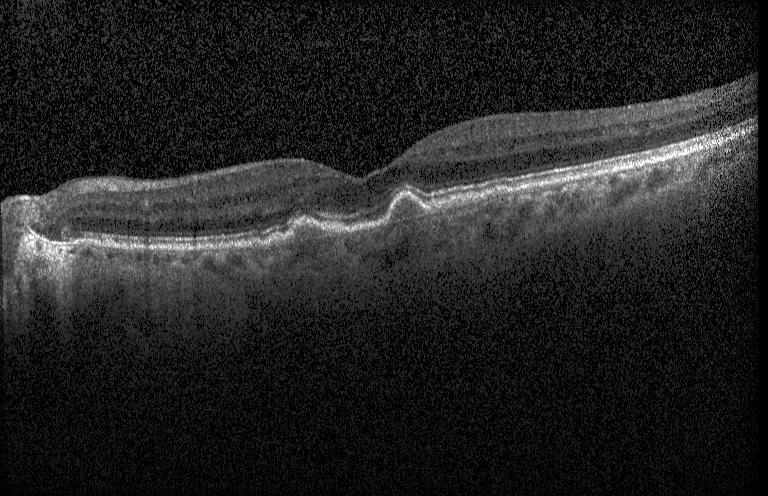
OCT line scan; Heidelberg Spectralis OCT system — Finding: drusen.